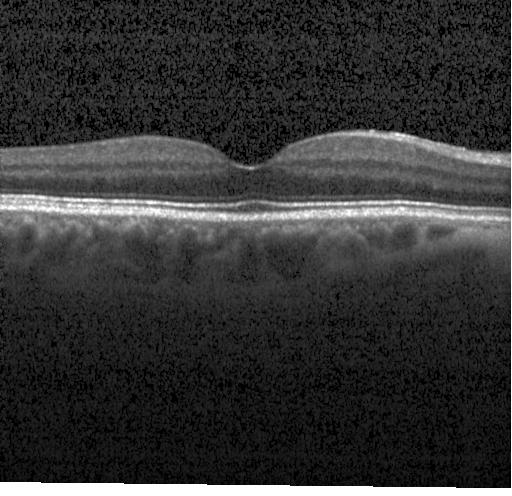
Finding: no evidence of CNV, DME, or drusen.